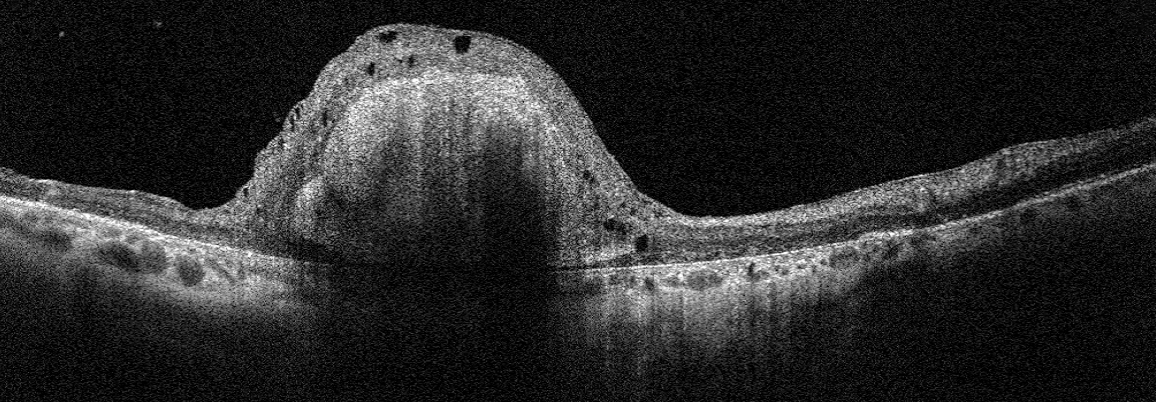 OCT B-scan · fovea-centered · instrument: Optovue Avanti RTVue XR — Impression: age-related macular degeneration.